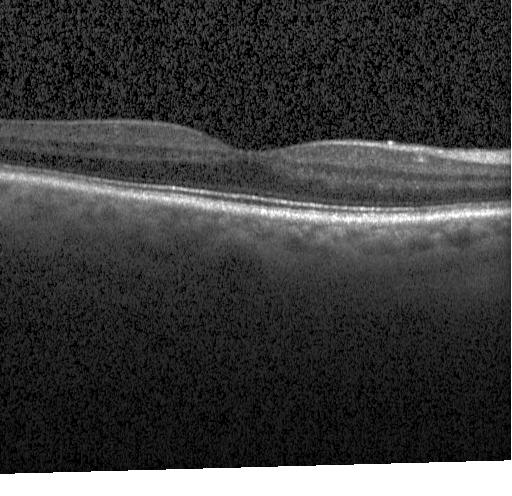

Retinal OCT cross-section — OCT finding: no CNV, DME, or drusen.